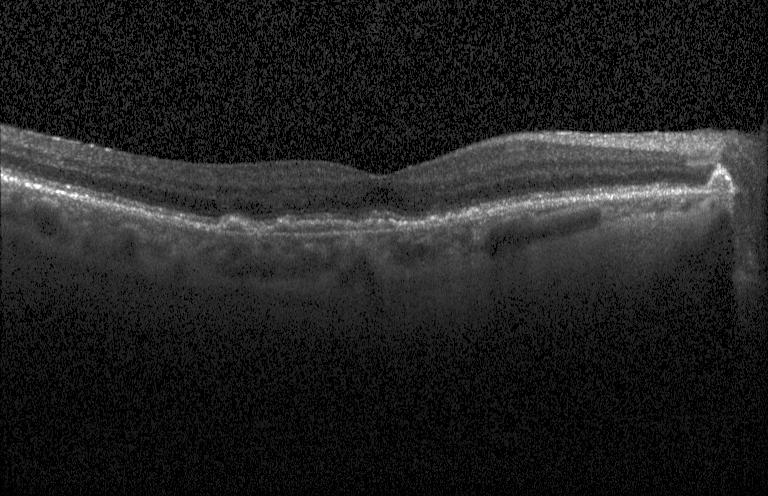 Macular scan, spectral-domain optical coherence tomography, OCT line scan, Heidelberg Spectralis OCT system.
A choroidal neovascular membrane.